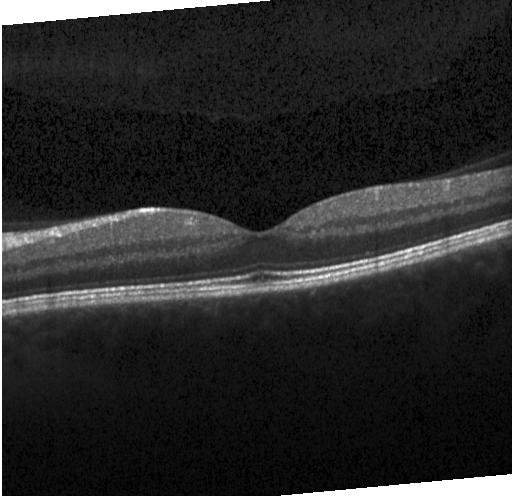

Retinal OCT cross-section showing no evidence of choroidal neovascularization, diabetic macular edema, or drusen.